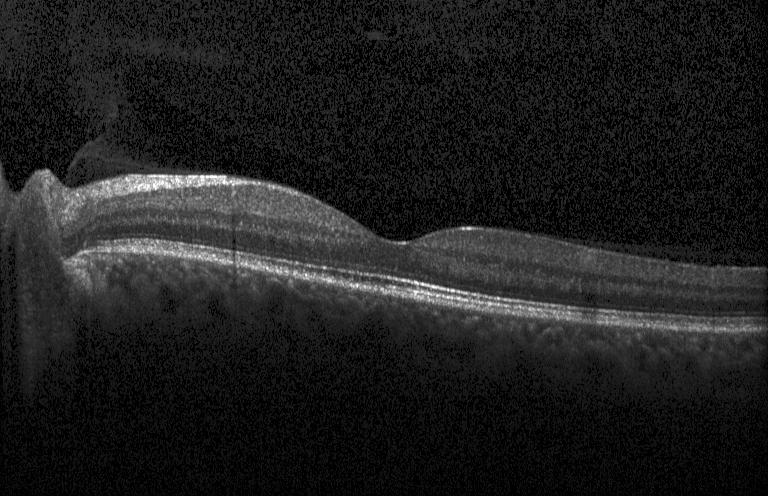 Optical coherence tomography B-scan
The scan shows no choroidal neovascularization, no diabetic macular edema, and no drusen.